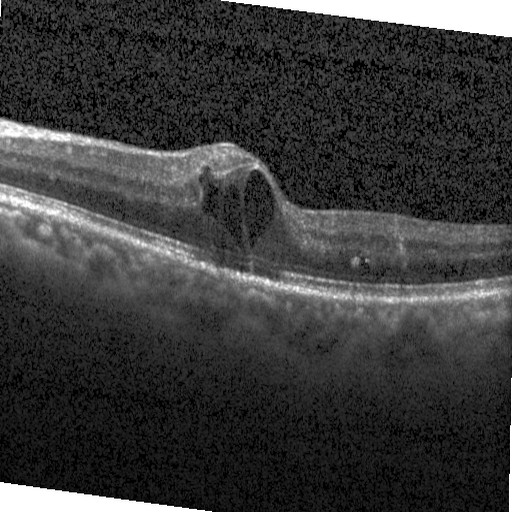

Optical coherence tomography B-scan, SD-OCT, Heidelberg Spectralis
Diabetic macular edema.